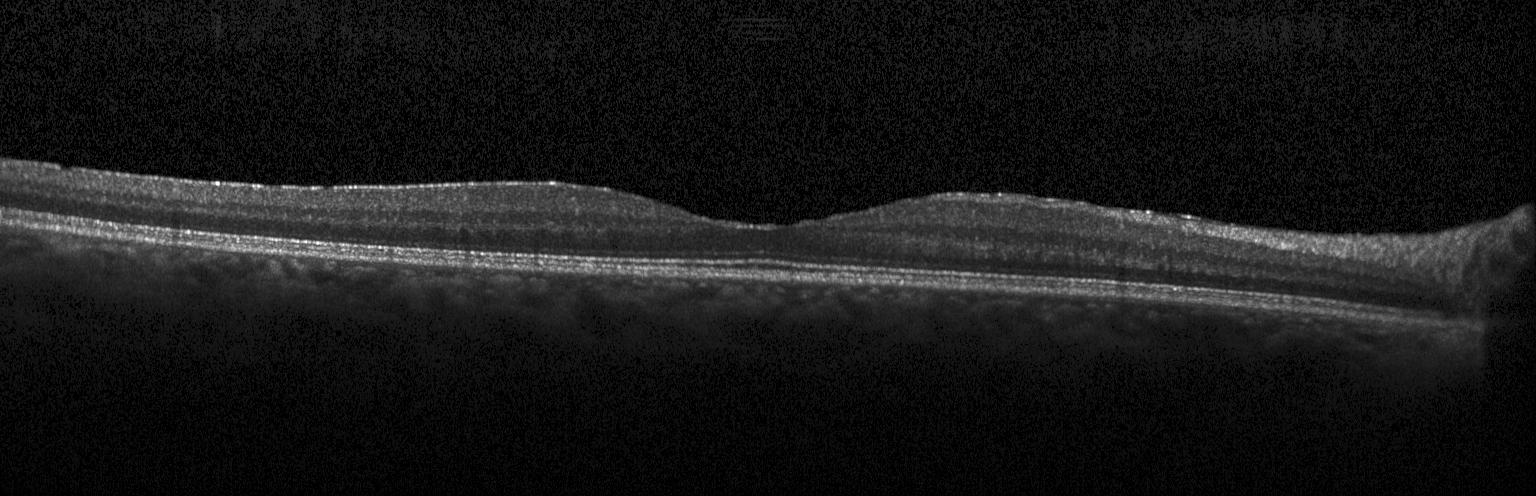 Impression: neither choroidal neovascularization, diabetic macular edema, nor drusen.